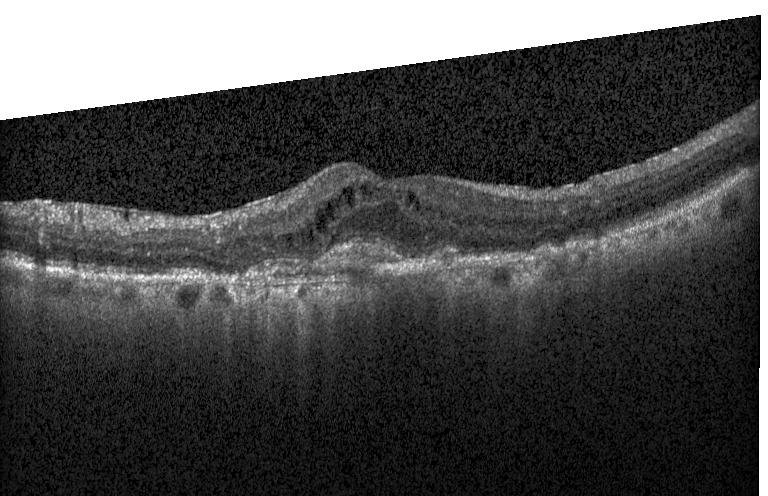
Retinal OCT cross-section showing a choroidal neovascular membrane.